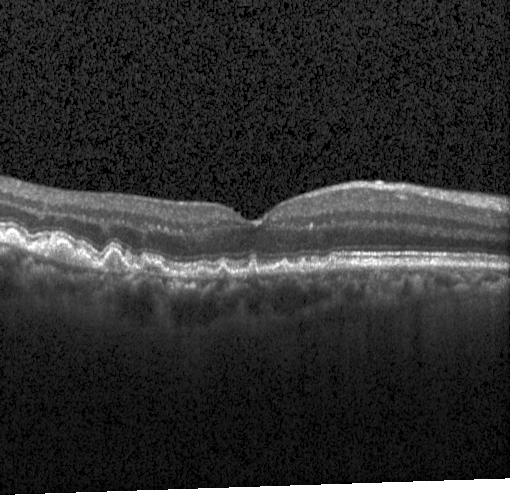

This B-scan demonstrates sub-RPE drusenoid deposits.